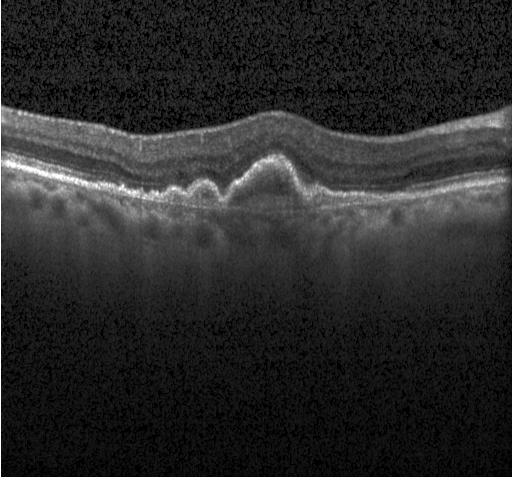

Retinal OCT B-scan; SD-OCT; instrument: Heidelberg Spectralis
This B-scan demonstrates a choroidal neovascular membrane.